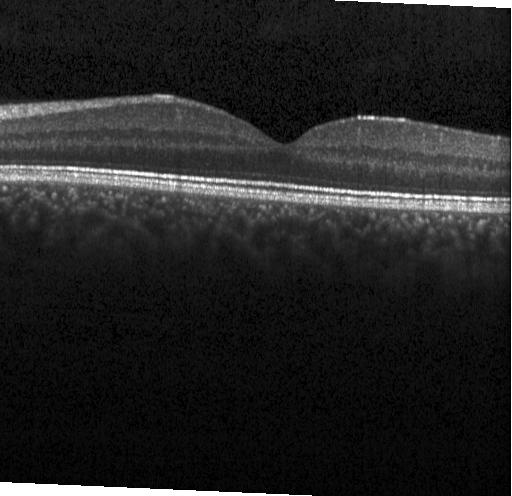 Retinal OCT cross-section showing no CNV, DME, or drusen.